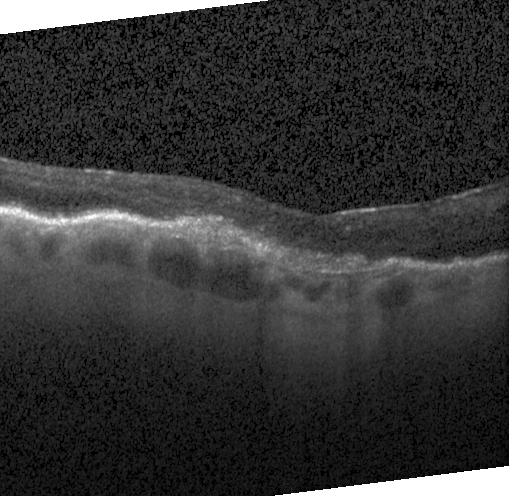 Macular OCT demonstrating choroidal neovascularization.